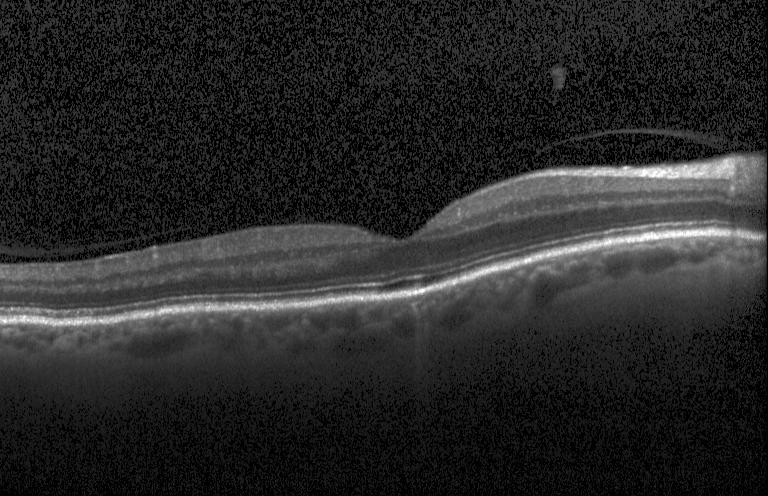
OCT line scan · Heidelberg Spectralis · spectral-domain optical coherence tomography · centered on the fovea.
Macular OCT: neither CNV, DME, nor drusen.